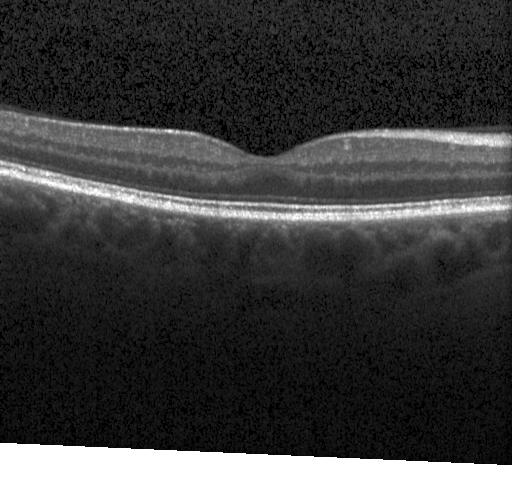 Macular OCT demonstrating no choroidal neovascularization, no diabetic macular edema, and no drusen.